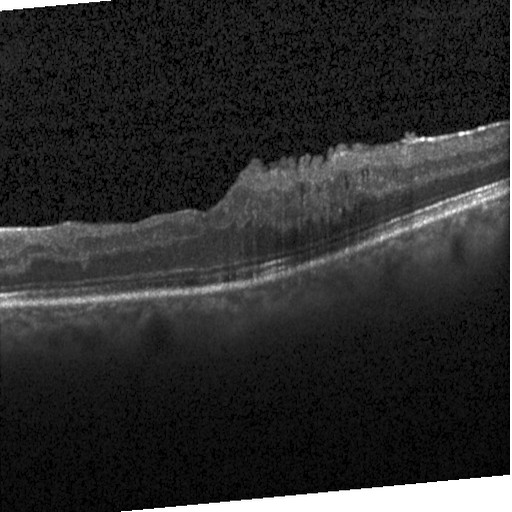

Assessment: diabetic macular edema.